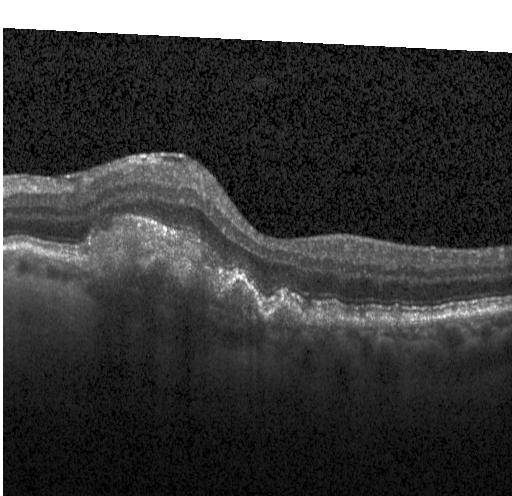
Acquired on a Heidelberg Spectralis, centered on the fovea, retinal OCT cross-section.
The scan shows choroidal neovascularization.